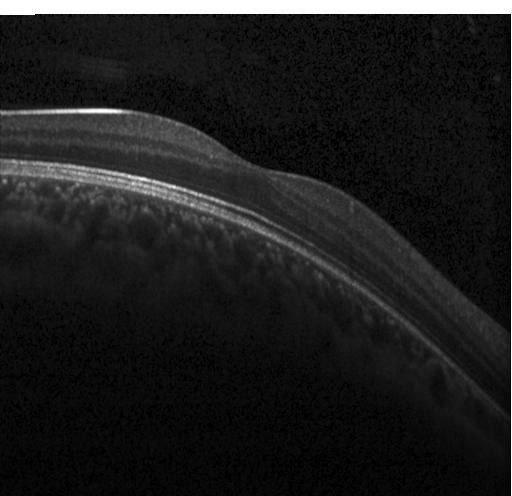 SD-OCT. Heidelberg Spectralis OCT system. Fovea-centered. Retinal OCT B-scan. Impression: no CNV, DME, or drusen.